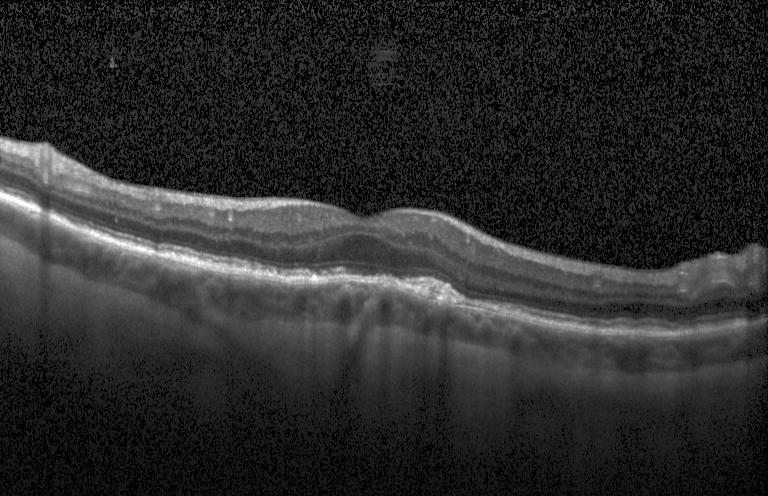 Heidelberg Spectralis. Fovea-centered. Spectral-domain OCT. Retinal OCT B-scan
Assessment: CNV.